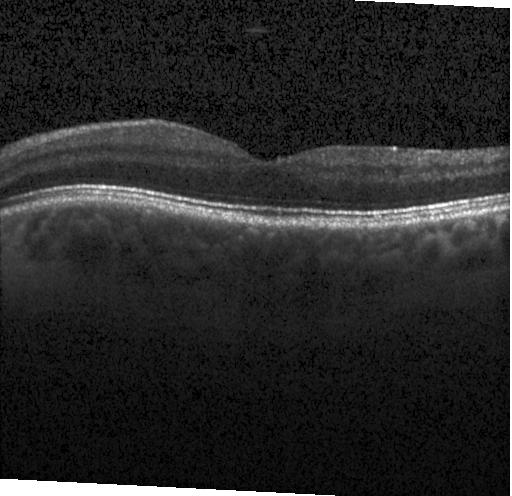

Finding: no CNV, DME, or drusen.